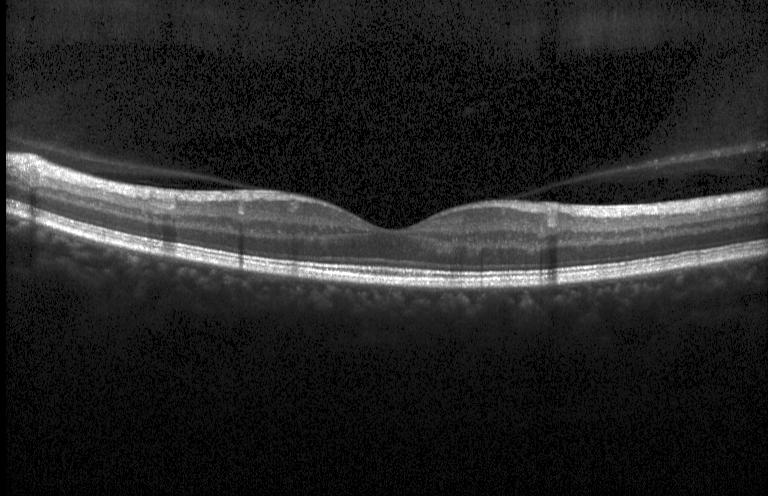 OCT B-scan, Heidelberg Spectralis, SD-OCT, horizontal scan through the fovea
No evidence of choroidal neovascularization, diabetic macular edema, or drusen.